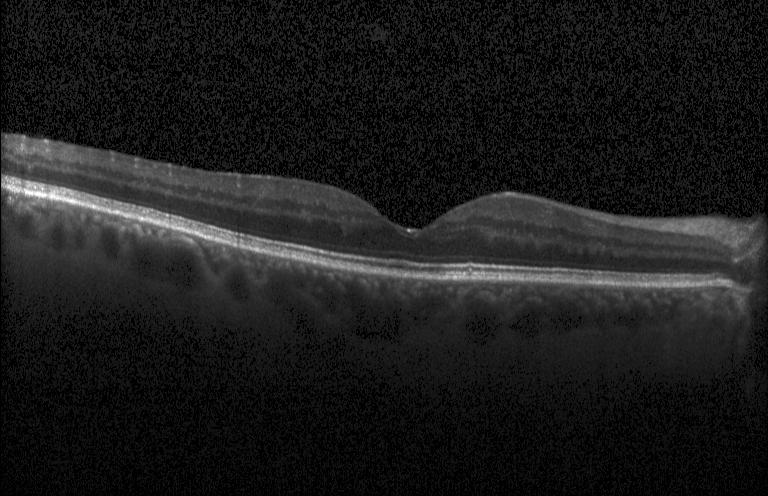
Centered on the fovea, spectral-domain OCT, retinal OCT cross-section, Heidelberg Spectralis OCT system.
Impression: no choroidal neovascularization, diabetic macular edema, or drusen.